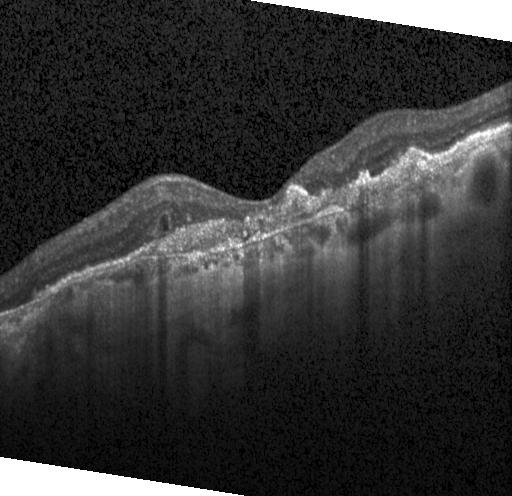
OCT line scan · macular scan. Diagnosis: a choroidal neovascular membrane.